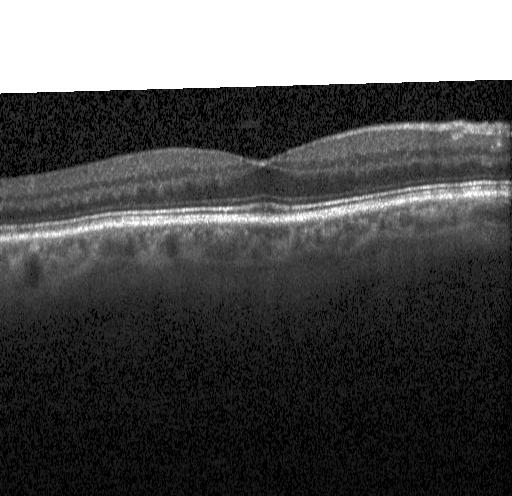
Heidelberg Spectralis OCT system, horizontal scan through the fovea, optical coherence tomography B-scan. Assessment: no CNV, no DME, and no drusen.